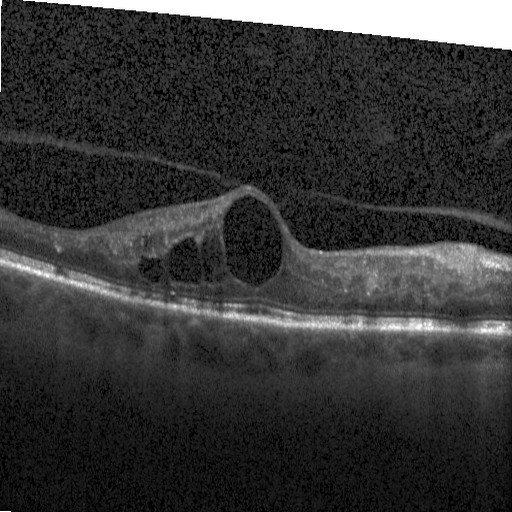

Retinal OCT B-scan — Impression: diabetic macular edema.